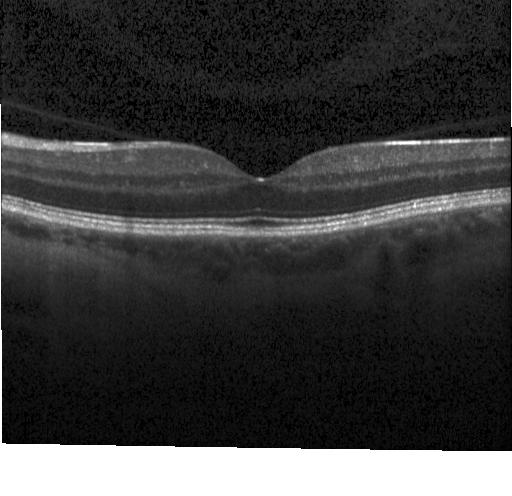 Fovea-centered · optical coherence tomography scan. Diagnosis: neither CNV, DME, nor drusen.